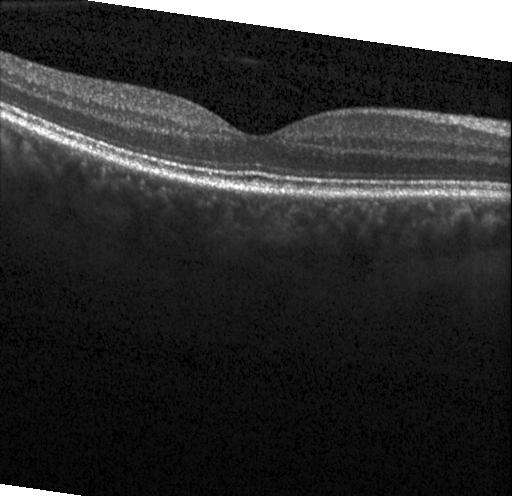

Diagnosis: no evidence of CNV, DME, or drusen.